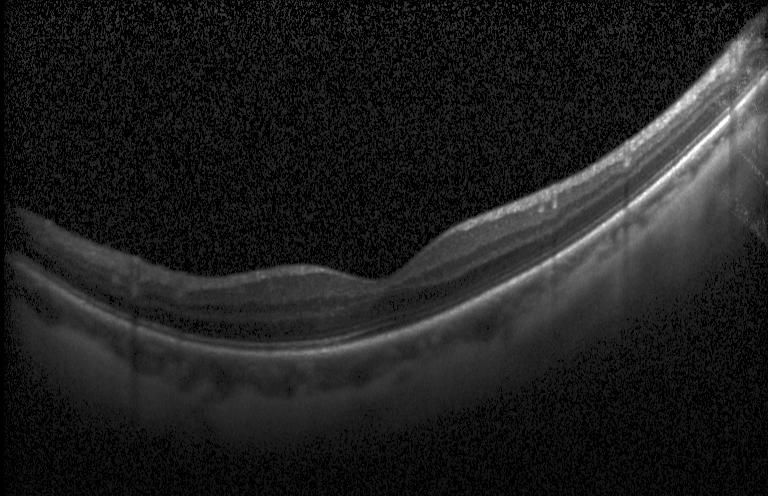
OCT B-scan showing no CNV, no DME, and no drusen.